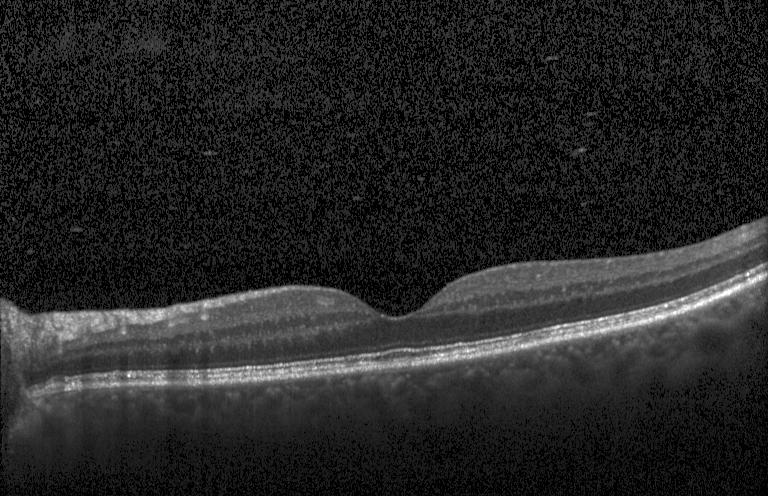 Retinal OCT cross-section. Impression: no choroidal neovascularization, diabetic macular edema, or drusen.